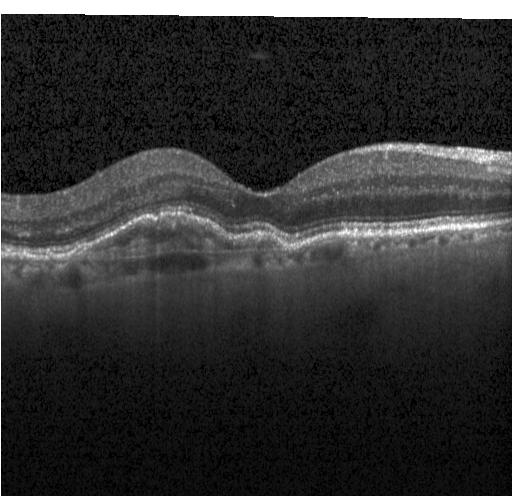
Retinal OCT cross-section, spectral-domain optical coherence tomography, fovea-centered, Heidelberg Spectralis OCT system.
Dx: a choroidal neovascular membrane.